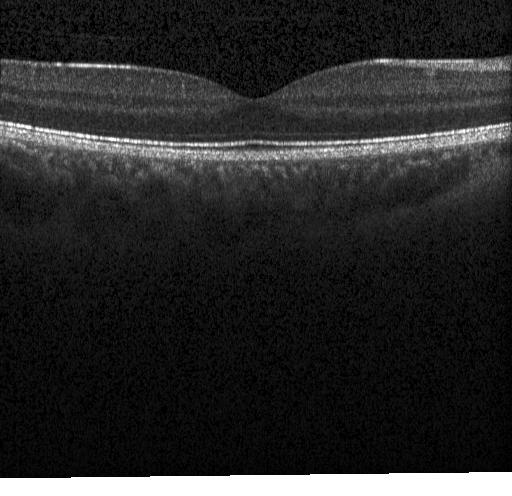
The scan shows no choroidal neovascularization, diabetic macular edema, or drusen.